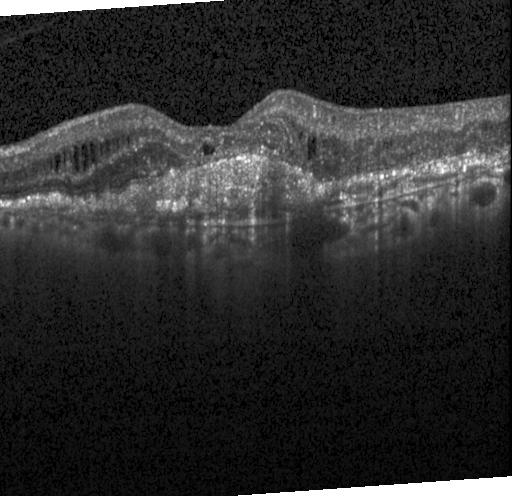

Optical coherence tomography scan
Macular OCT: choroidal neovascularization (CNV).